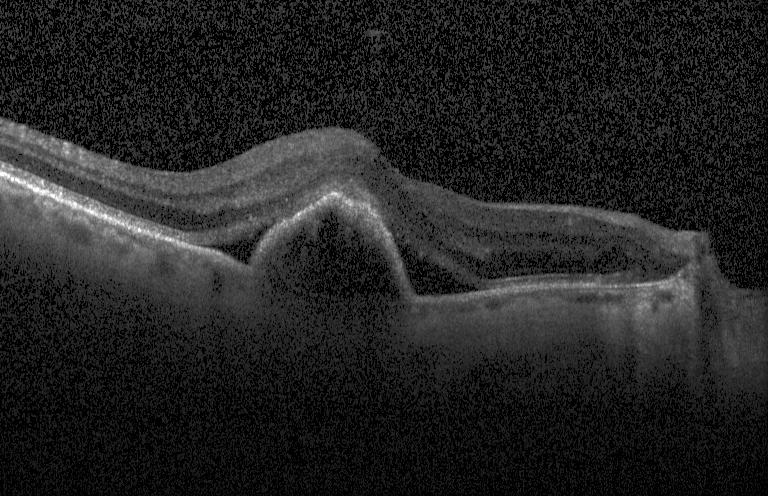
Fovea-centered, spectral-domain optical coherence tomography, optical coherence tomography scan, instrument: Heidelberg Spectralis
Impression: choroidal neovascularization (CNV).